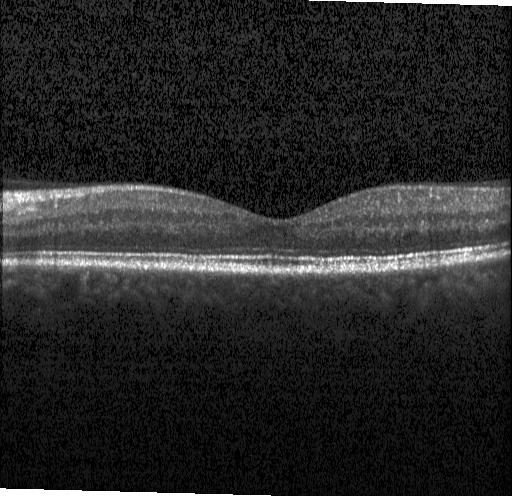 OCT B-scan showing neither choroidal neovascularization, diabetic macular edema, nor drusen.